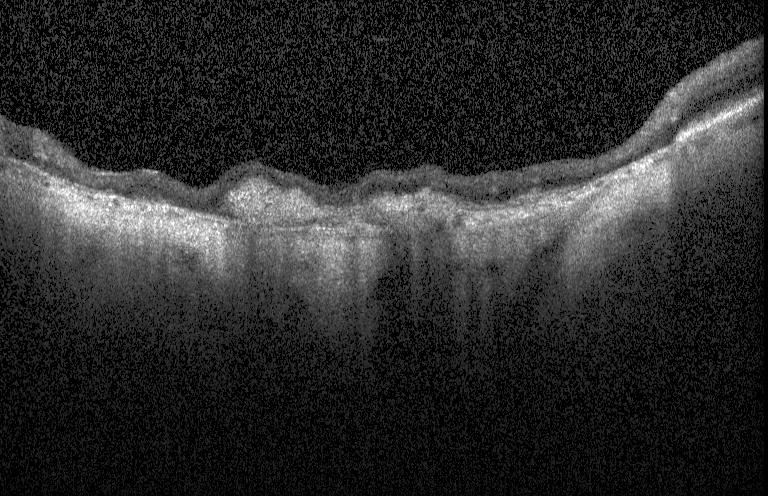
Impression: CNV.